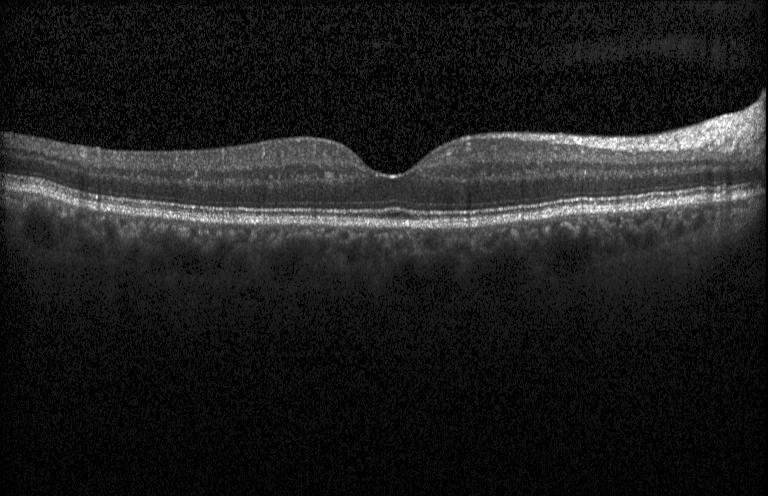

Finding: no choroidal neovascularization, diabetic macular edema, or drusen.